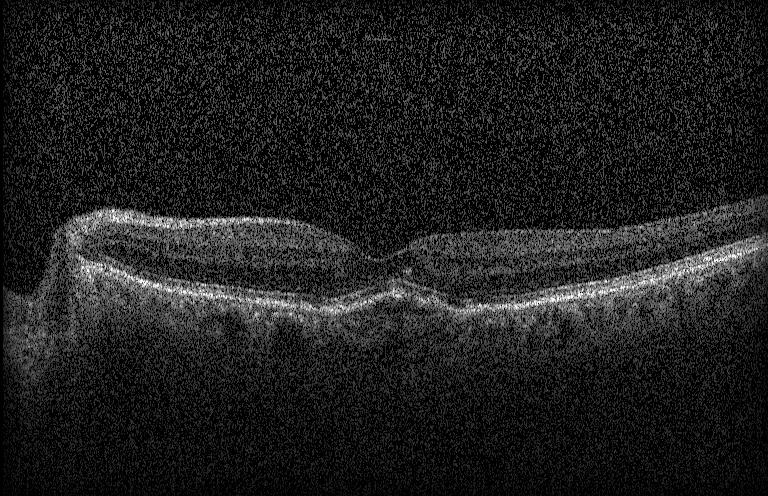

OCT finding: a choroidal neovascular membrane.